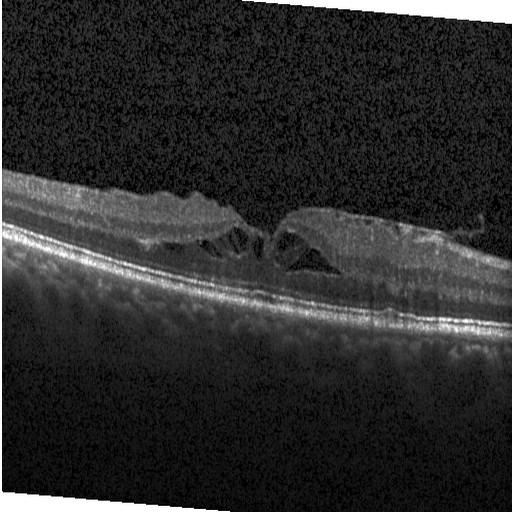 OCT line scan, spectral-domain OCT
Macular OCT: diabetic macular edema (DME).